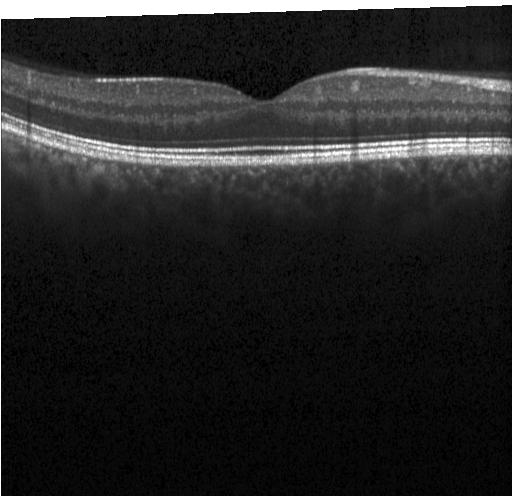
Retinal OCT cross-section · SD-OCT. Diagnosis: no evidence of choroidal neovascularization, diabetic macular edema, or drusen.